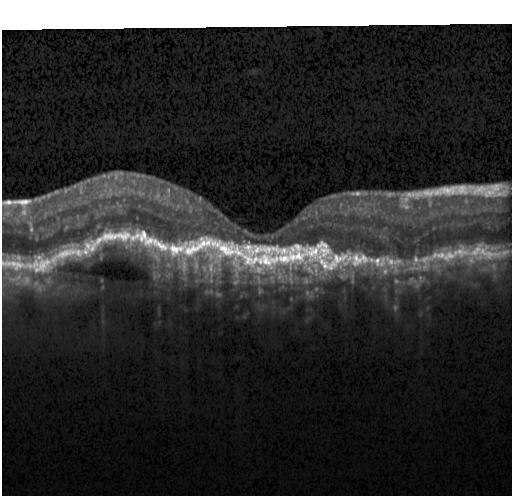

Optical coherence tomography B-scan; acquired on a Heidelberg Spectralis; centered on the fovea; SD-OCT
Macular OCT: choroidal neovascularization.